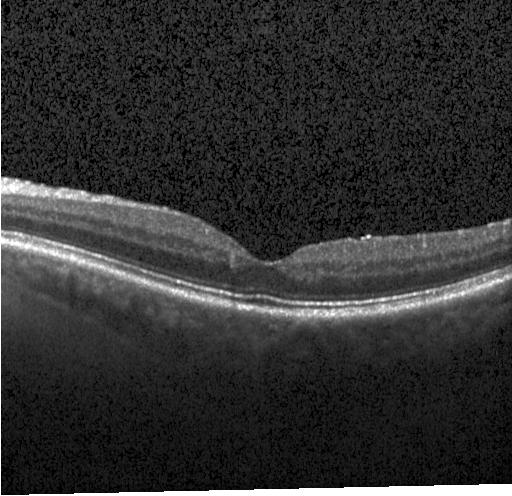

Retinal OCT cross-section. Spectral-domain optical coherence tomography.
Dx: neither choroidal neovascularization, diabetic macular edema, nor drusen.